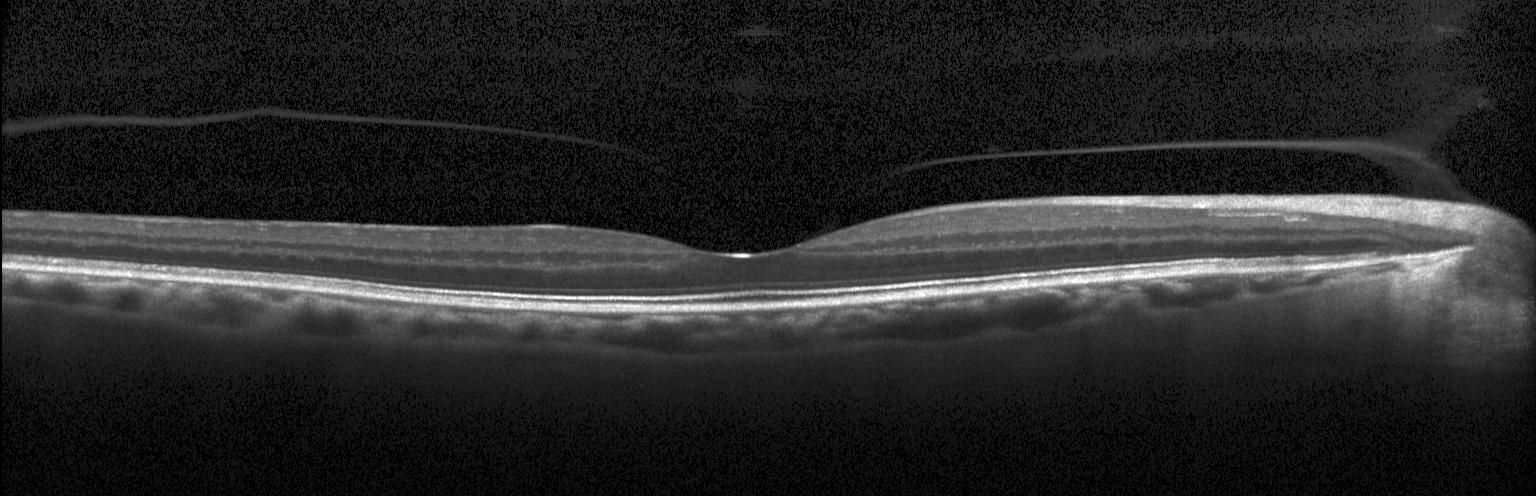

The scan shows no CNV, DME, or drusen.